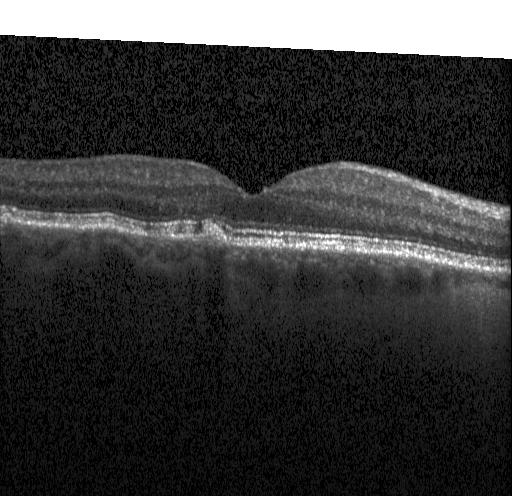
Multiple drusen.